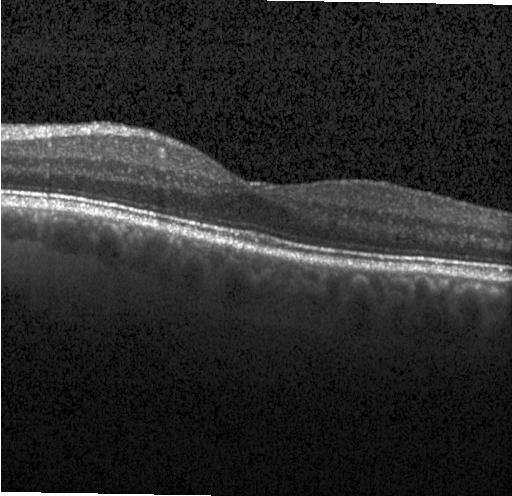
Retinal OCT B-scan. Horizontal scan through the fovea. Diagnosis: no evidence of choroidal neovascularization, diabetic macular edema, or drusen.